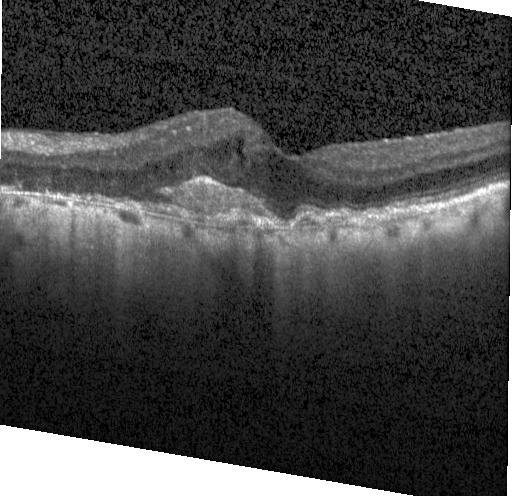
Instrument: Heidelberg Spectralis · OCT B-scan · through the macula · spectral-domain optical coherence tomography.
Impression: choroidal neovascularization (CNV).